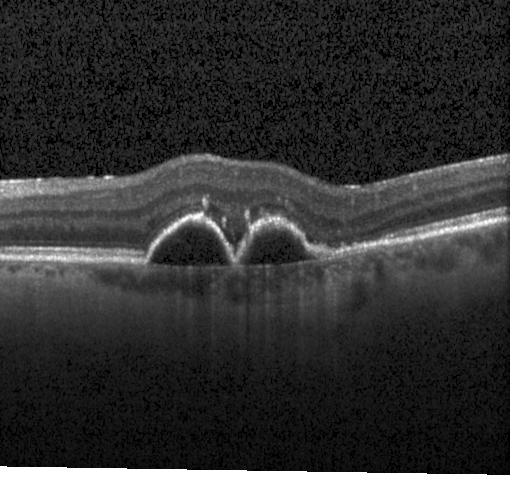

OCT scan showing a choroidal neovascular membrane.